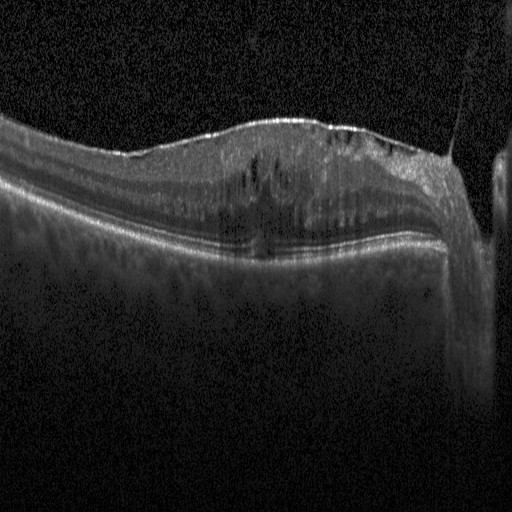 OCT B-scan showing diabetic macular edema.